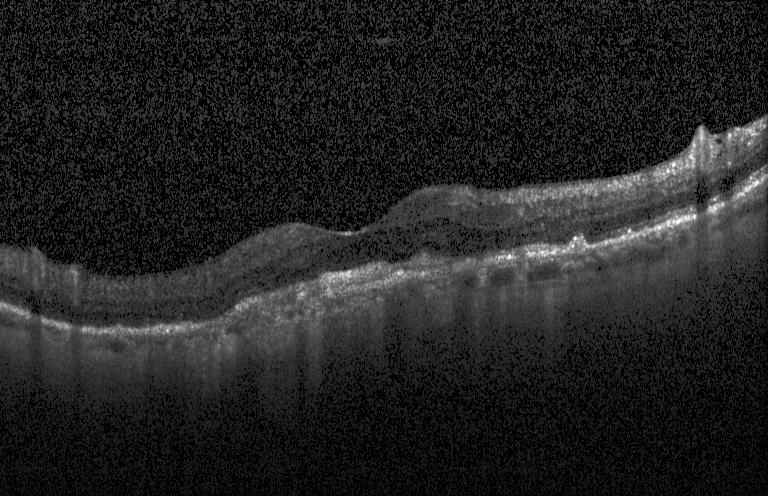

SD-OCT; Heidelberg Spectralis; retinal OCT B-scan — Diagnosis: a choroidal neovascular membrane.